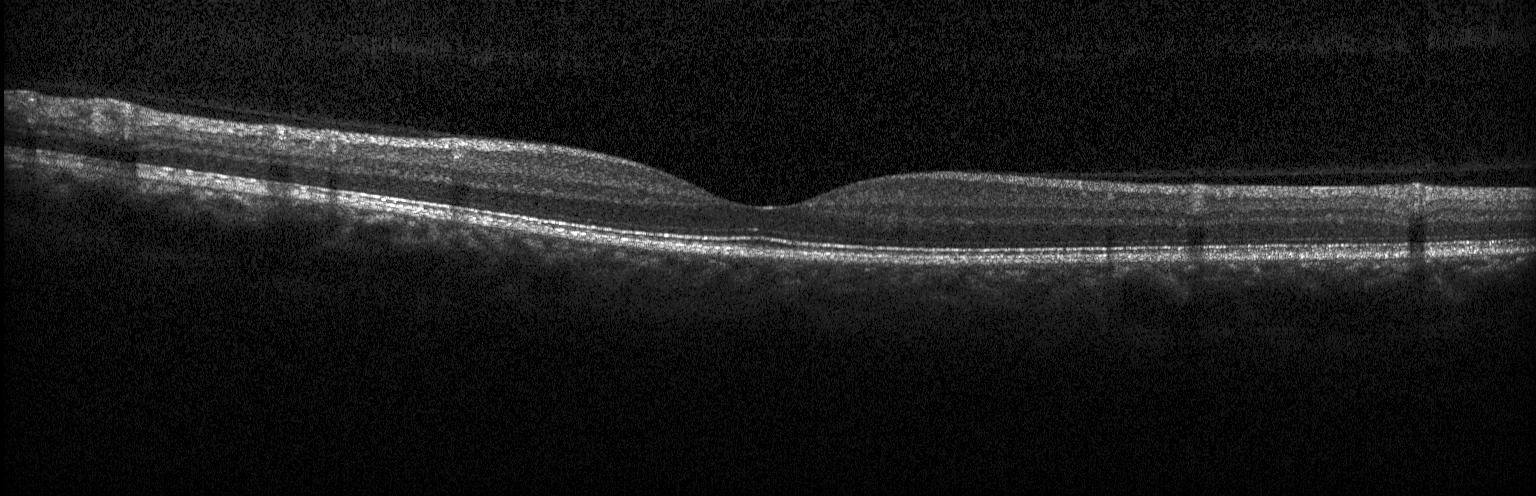 OCT B-scan, macular scan, SD-OCT, instrument: Heidelberg Spectralis — Macular OCT: no choroidal neovascularization, diabetic macular edema, or drusen.